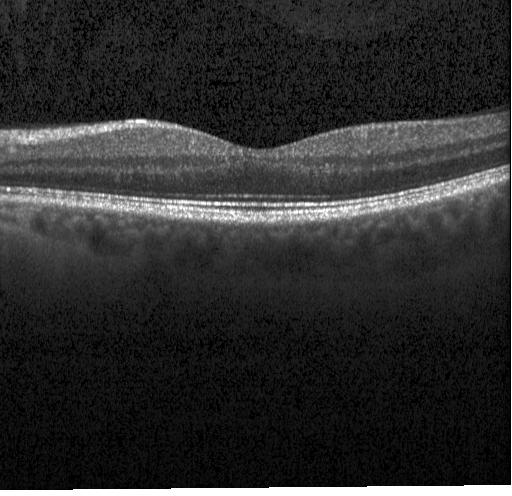 Optical coherence tomography scan, spectral-domain OCT, through the macula — Assessment: no choroidal neovascularization, diabetic macular edema, or drusen.